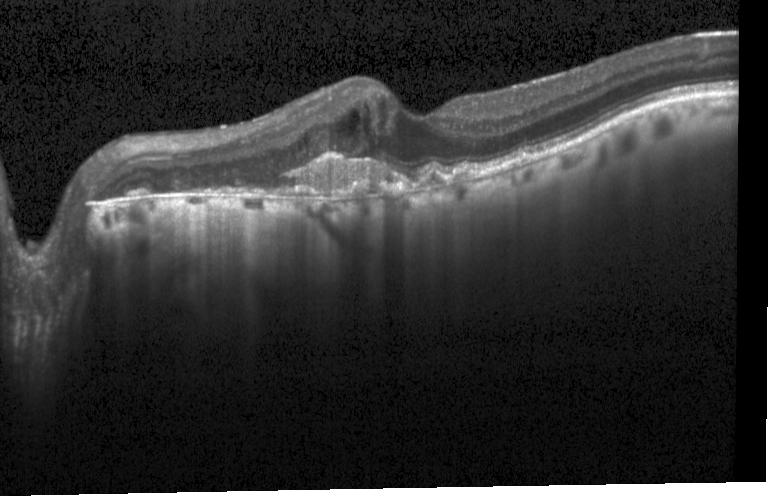 Optical coherence tomography scan · instrument: Heidelberg Spectralis. Assessment: a choroidal neovascular membrane.